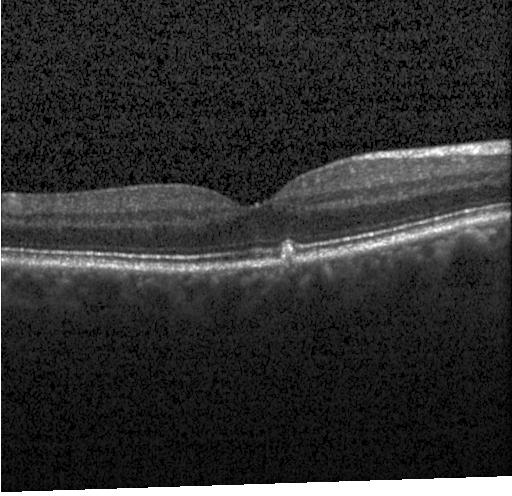
Optical coherence tomography B-scan. The scan shows sub-RPE drusenoid deposits.